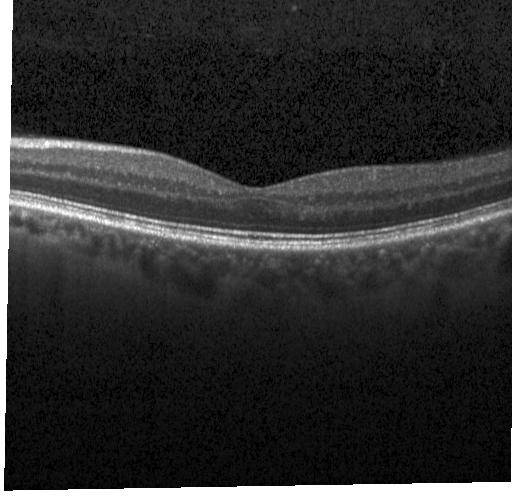
Macular scan. SD-OCT. Optical coherence tomography scan.
Assessment: no choroidal neovascularization, no diabetic macular edema, and no drusen.